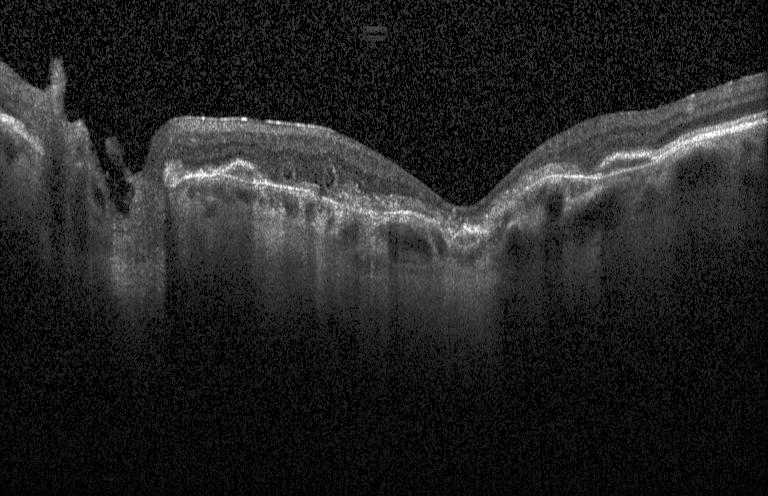

Optical coherence tomography scan · instrument: Heidelberg Spectralis · SD-OCT
CNV.